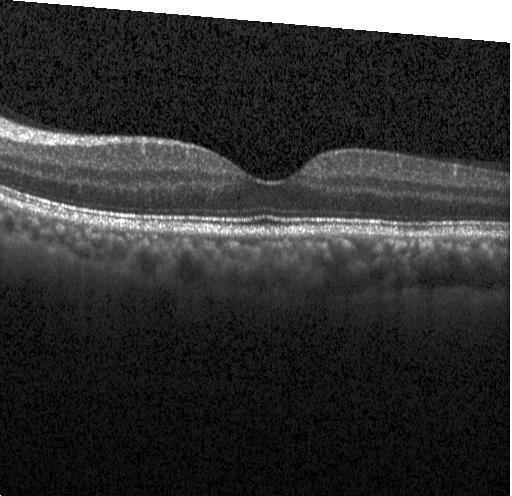

Retinal OCT B-scan, SD-OCT, acquired on a Heidelberg Spectralis, fovea-centered
Finding: no choroidal neovascularization, diabetic macular edema, or drusen.